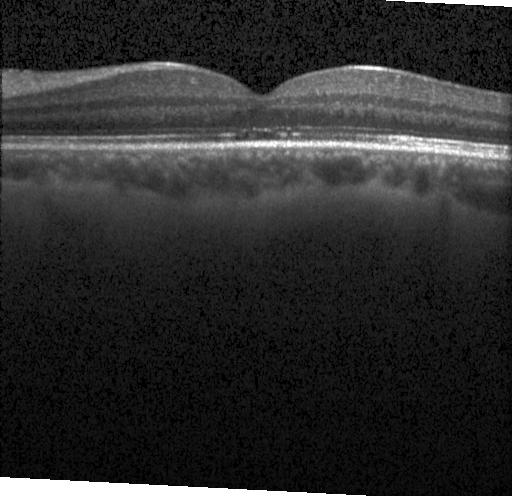
OCT line scan — Finding: neither CNV, DME, nor drusen.